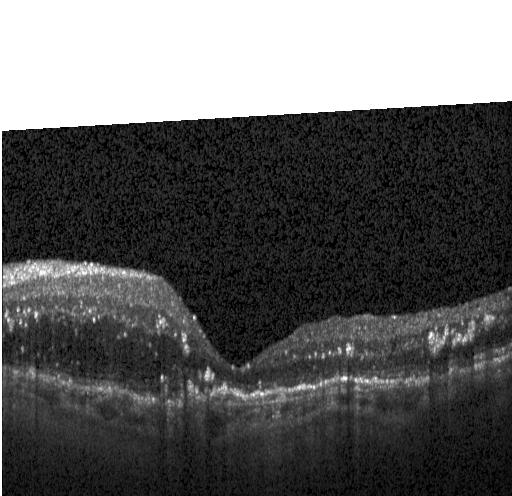
Diagnosis: CNV.